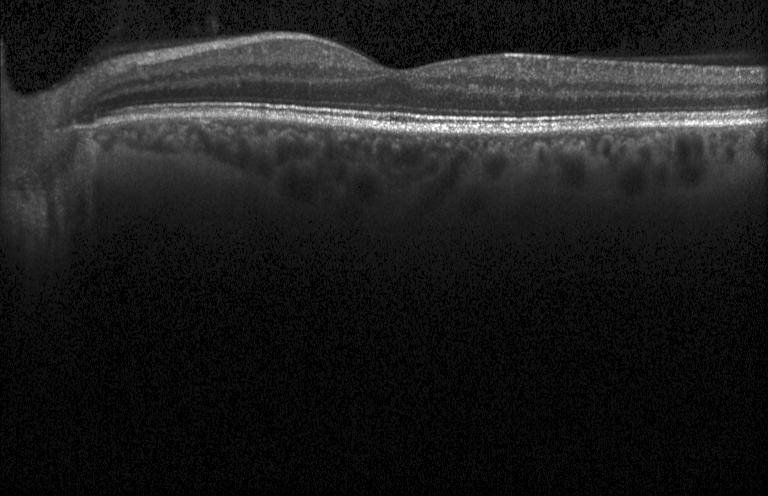 SD-OCT; acquired on a Heidelberg Spectralis; macular scan; optical coherence tomography scan.
Impression: no choroidal neovascularization, diabetic macular edema, or drusen.